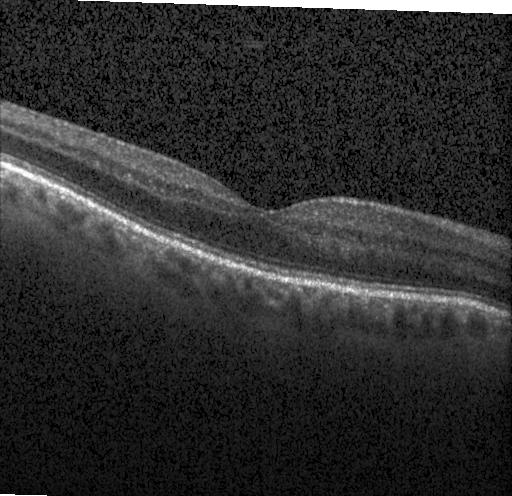
Heidelberg Spectralis OCT system · spectral-domain OCT · through the macula · retinal OCT cross-section
Diagnosis: no CNV, no DME, and no drusen.